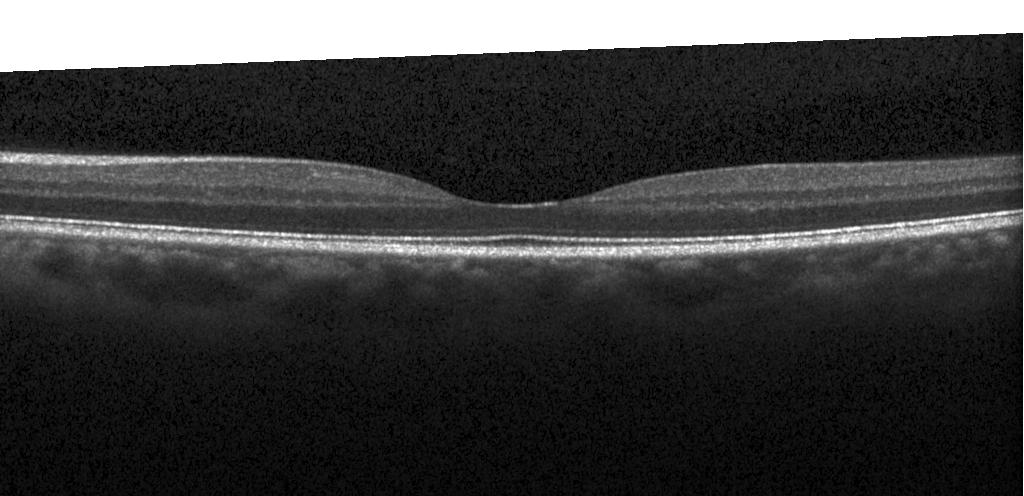

Retinal OCT B-scan.
The scan shows no choroidal neovascularization, diabetic macular edema, or drusen.